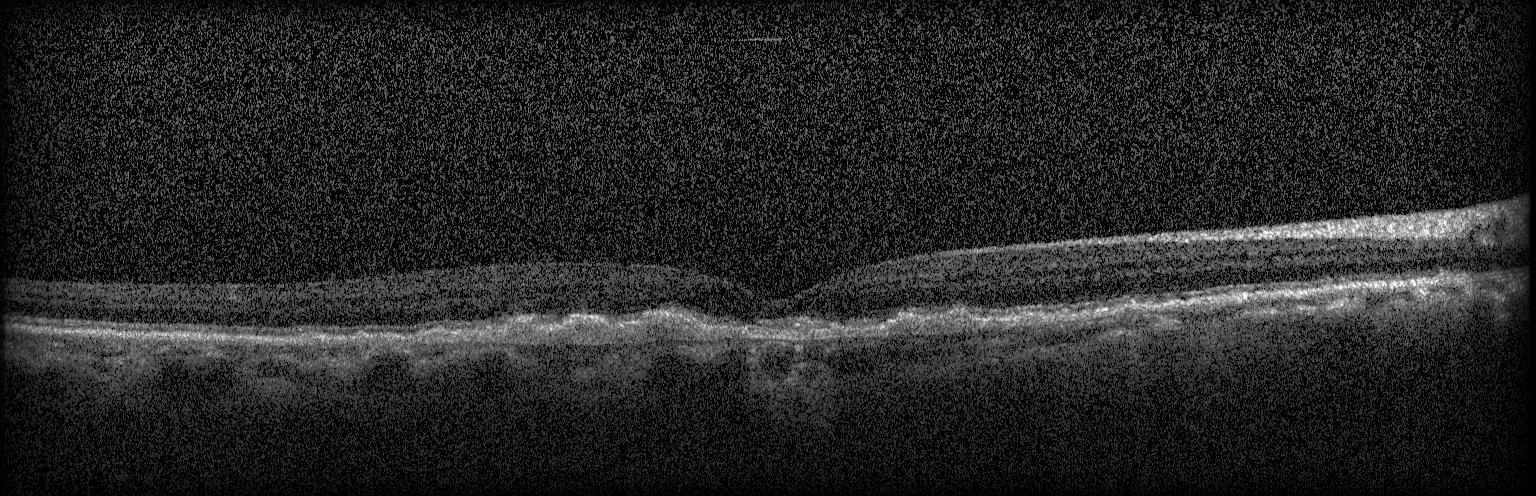
Macular scan. Instrument: Heidelberg Spectralis. SD-OCT. Retinal OCT B-scan — Dx: choroidal neovascularization (CNV).